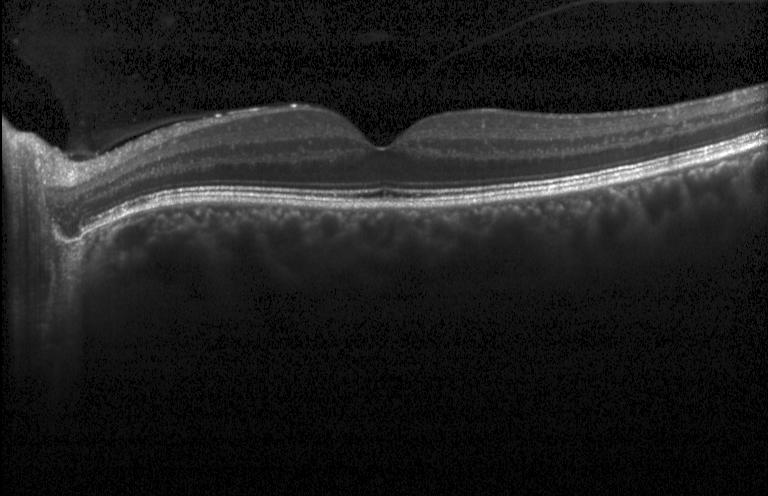

Finding: no choroidal neovascularization, no diabetic macular edema, and no drusen.